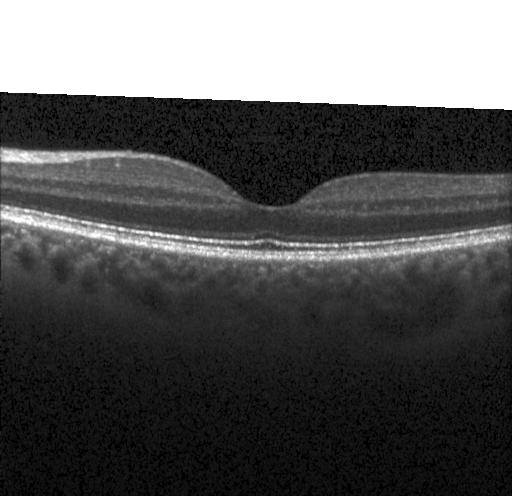 Impression: no evidence of choroidal neovascularization, diabetic macular edema, or drusen.